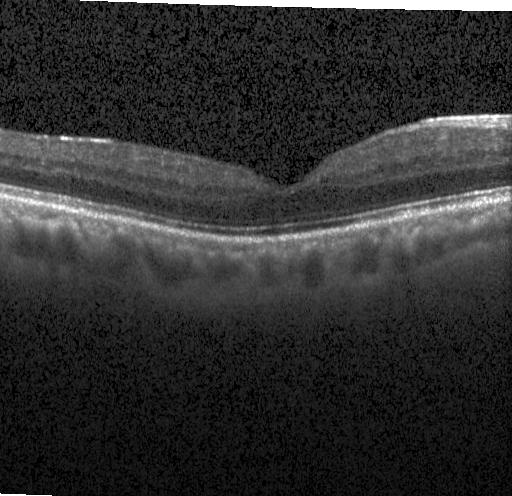 OCT finding: neither choroidal neovascularization, diabetic macular edema, nor drusen.